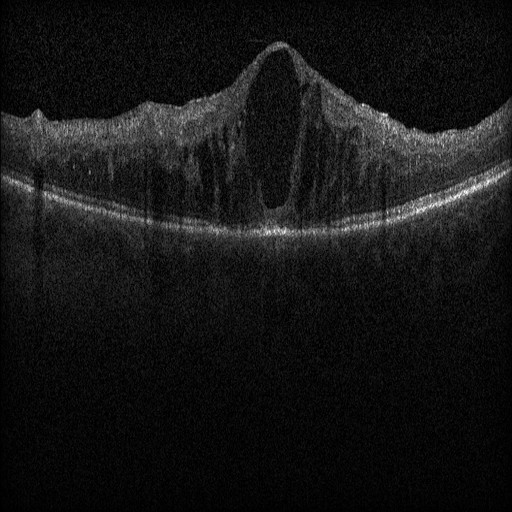
Retinal OCT B-scan — Diagnosis: diabetic macular edema.